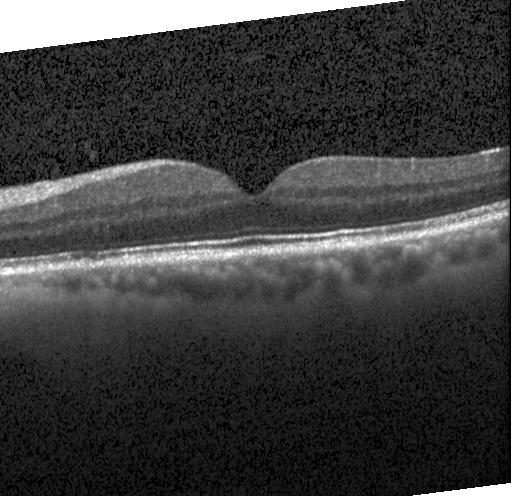 SD-OCT. OCT B-scan.
No choroidal neovascularization, diabetic macular edema, or drusen.